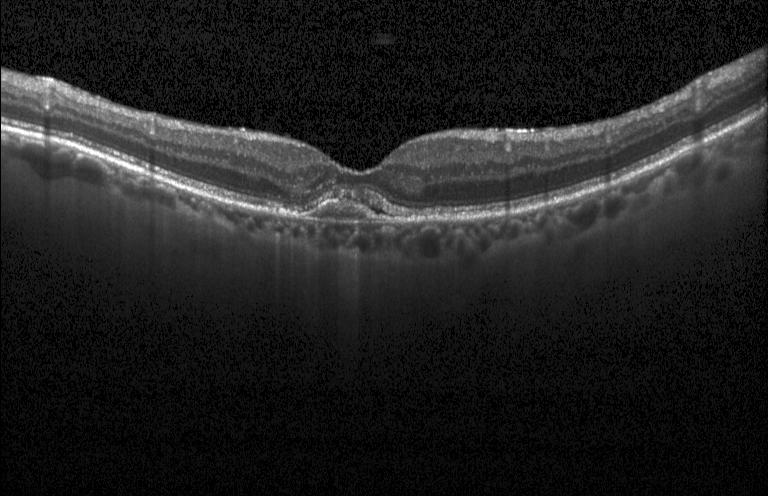
The scan shows a choroidal neovascular membrane.